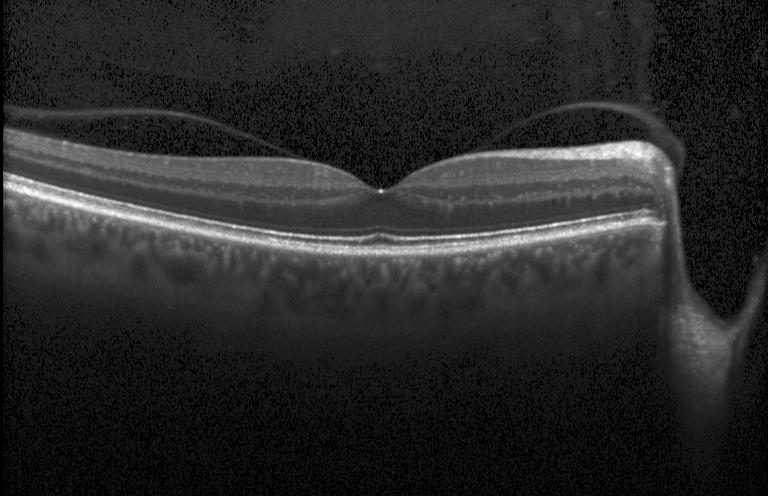 Spectral-domain OCT · macular scan · optical coherence tomography B-scan — Finding: no choroidal neovascularization, no diabetic macular edema, and no drusen.